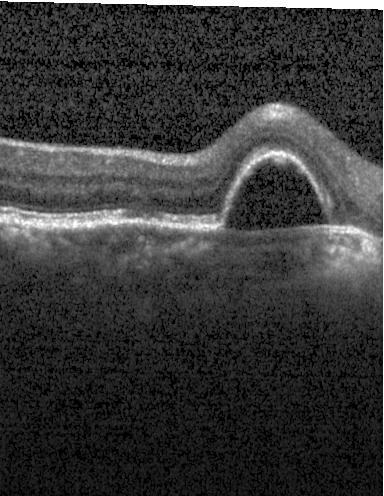
This B-scan demonstrates choroidal neovascularization (CNV).